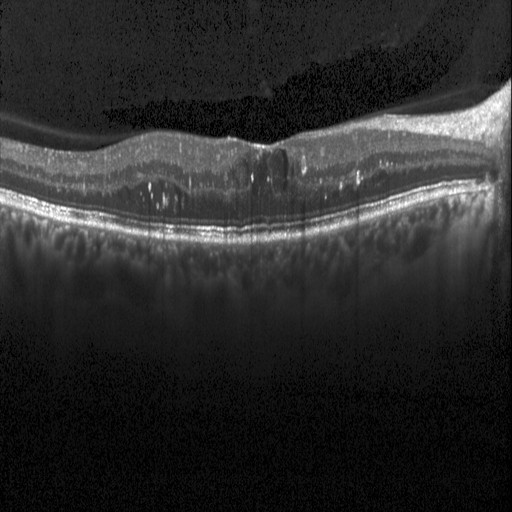
Spectral-domain optical coherence tomography, optical coherence tomography B-scan, Heidelberg Spectralis.
Assessment: diabetic macular edema.